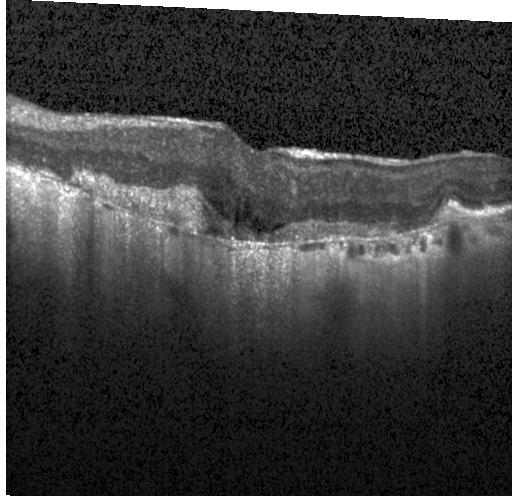
Assessment: a choroidal neovascular membrane.